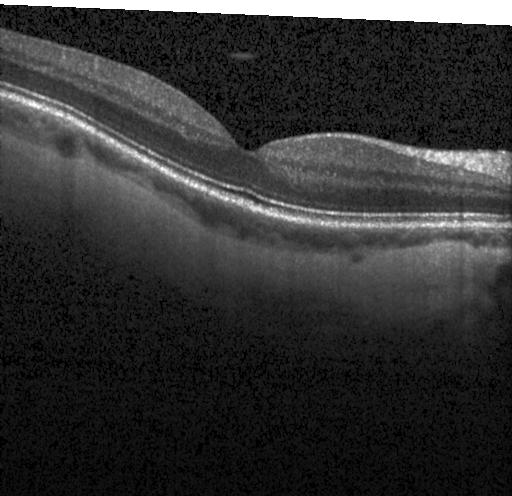

Centered on the fovea · OCT line scan · spectral-domain optical coherence tomography · Heidelberg Spectralis
Assessment: no CNV, no DME, and no drusen.